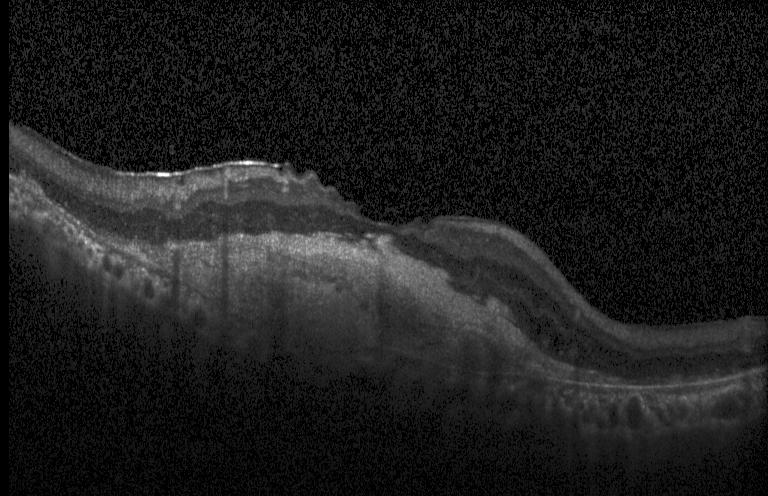 Heidelberg Spectralis OCT system · retinal OCT B-scan
Impression: a choroidal neovascular membrane.